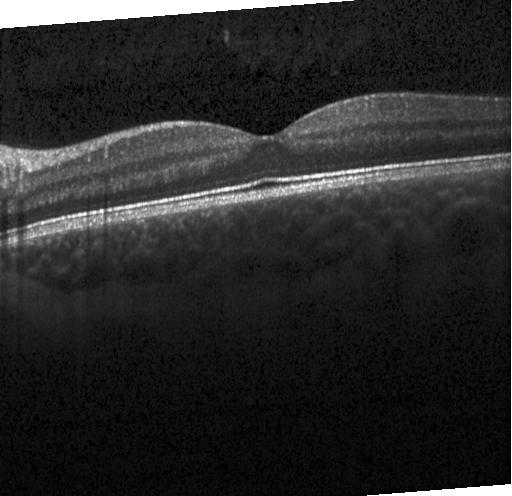 Spectral-domain OCT B-scan: no CNV, no DME, and no drusen.